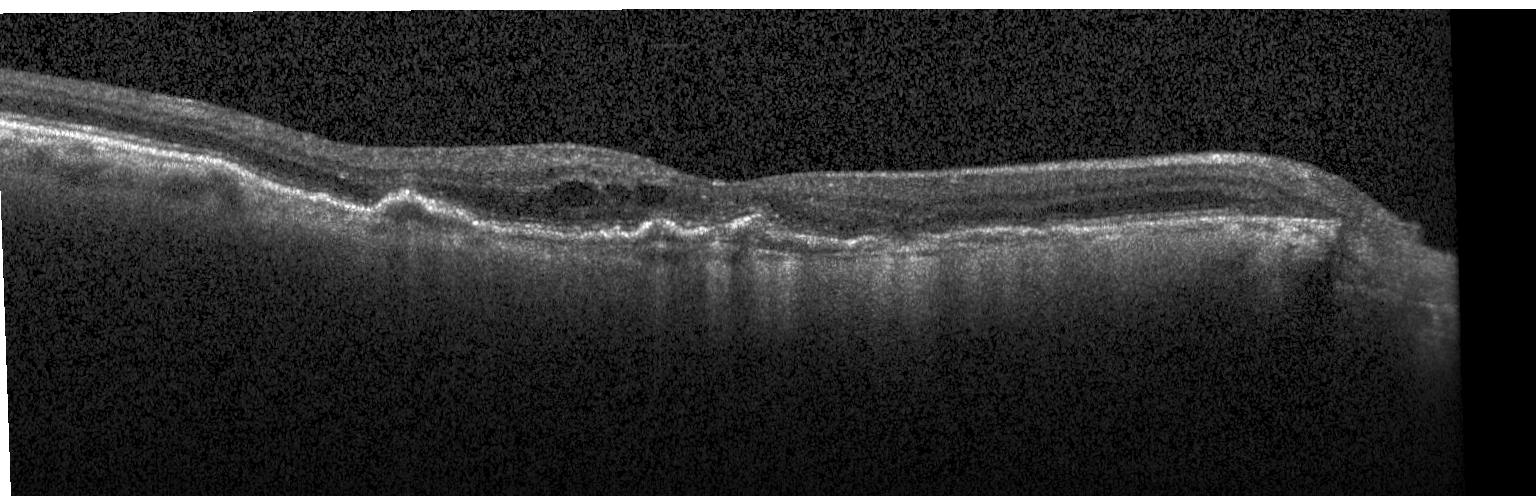

Spectral-domain OCT, through the macula, retinal OCT B-scan, Heidelberg Spectralis OCT system
OCT finding: CNV.